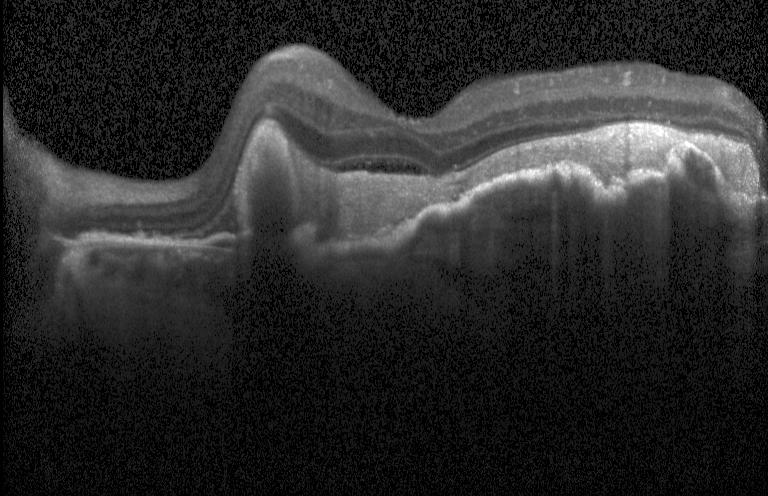
Fovea-centered; retinal OCT B-scan
The scan shows choroidal neovascularization.